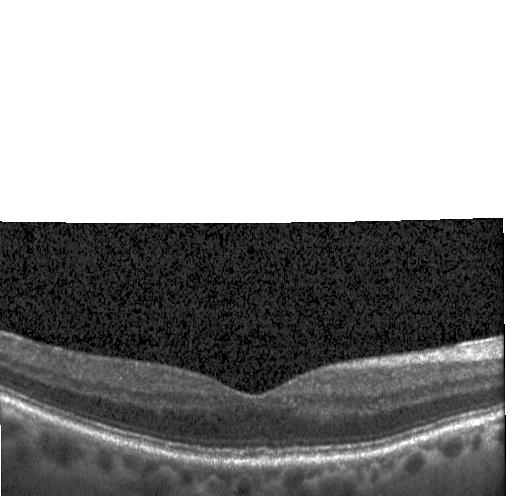 OCT B-scan · Heidelberg Spectralis · horizontal scan through the fovea · SD-OCT — This B-scan demonstrates no CNV, DME, or drusen.